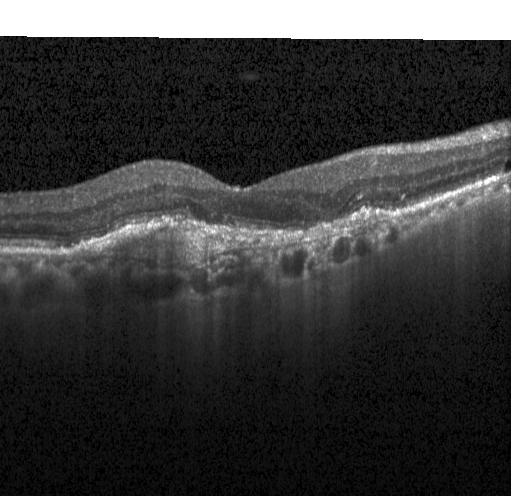 Fovea-centered · spectral-domain optical coherence tomography · instrument: Heidelberg Spectralis · retinal OCT B-scan.
Assessment: a choroidal neovascular membrane.